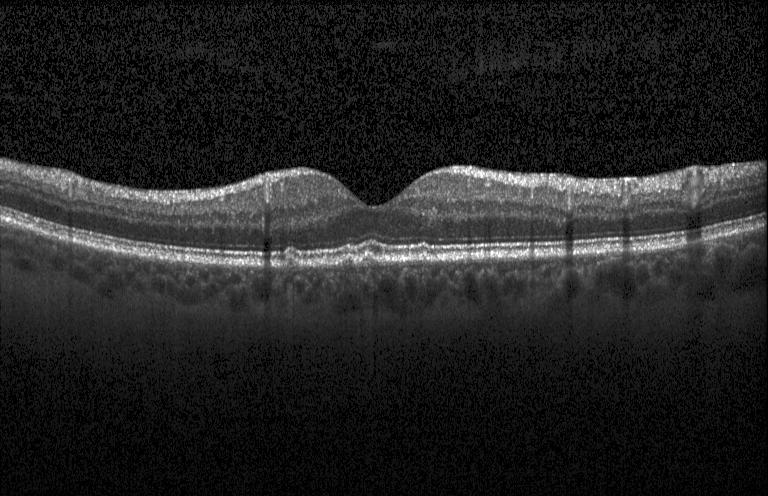 Heidelberg Spectralis · optical coherence tomography scan · horizontal scan through the fovea — Macular OCT: sub-RPE drusenoid deposits.